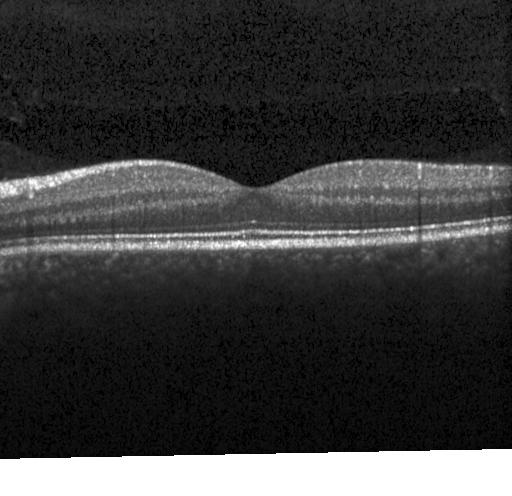
This B-scan demonstrates no evidence of choroidal neovascularization, diabetic macular edema, or drusen.